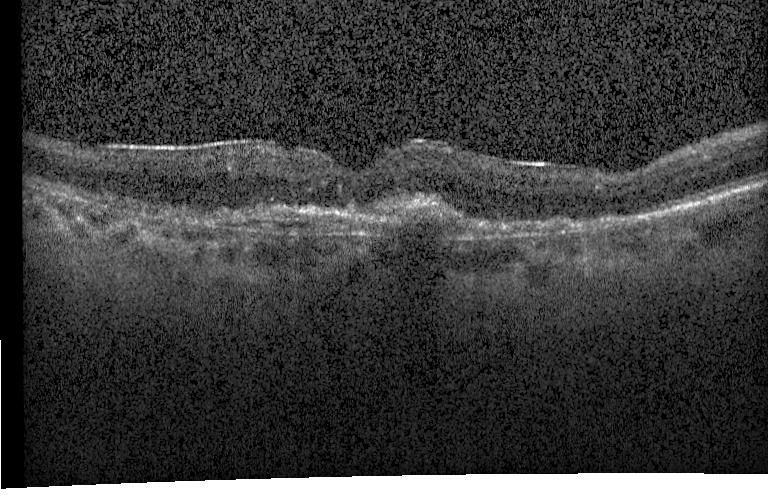
Horizontal scan through the fovea · OCT line scan — Finding: CNV.